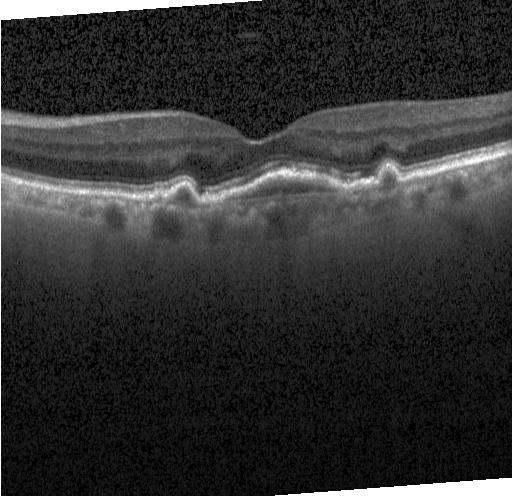
Diagnosis: CNV.